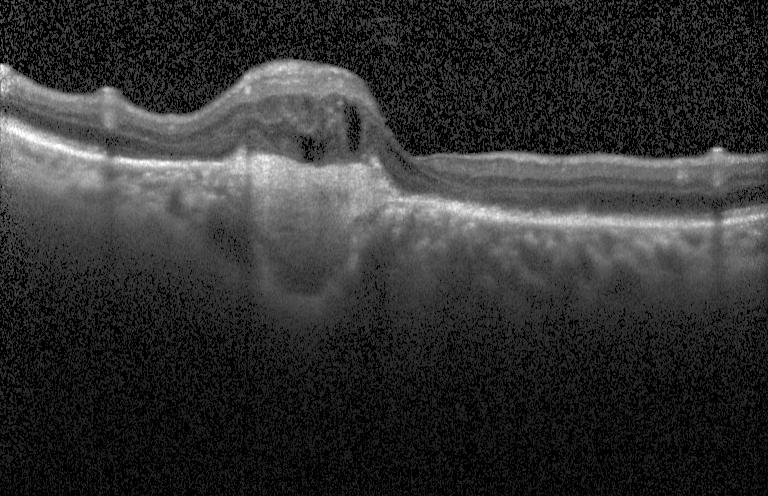
Impression: a choroidal neovascular membrane.